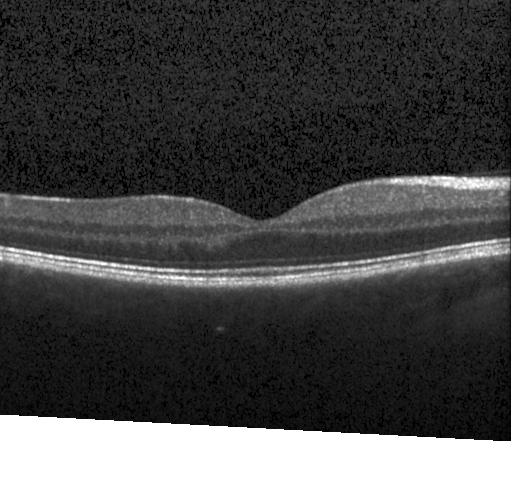

OCT scan showing no evidence of choroidal neovascularization, diabetic macular edema, or drusen.